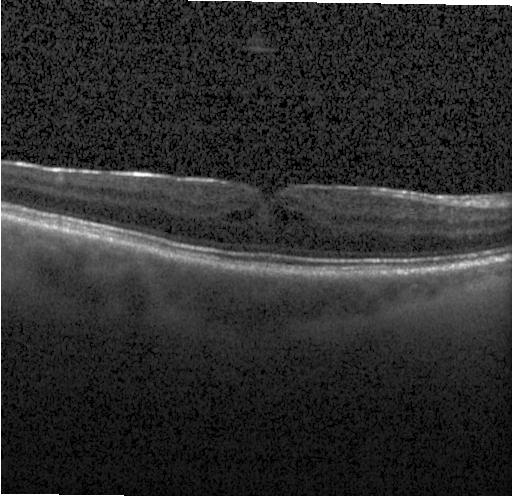

Acquired on a Heidelberg Spectralis, OCT line scan, centered on the fovea. OCT finding: DME.